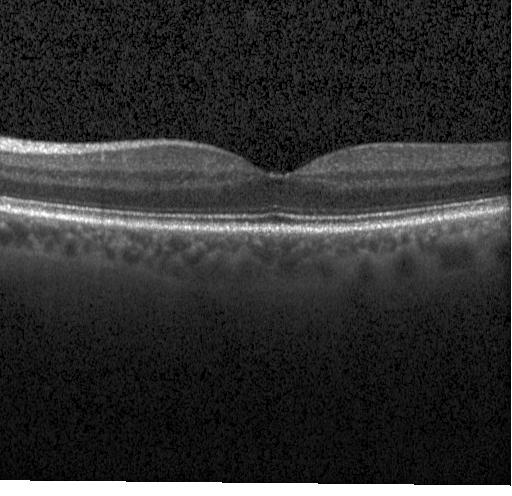
Heidelberg Spectralis OCT system; optical coherence tomography B-scan; SD-OCT
Assessment: neither CNV, DME, nor drusen.